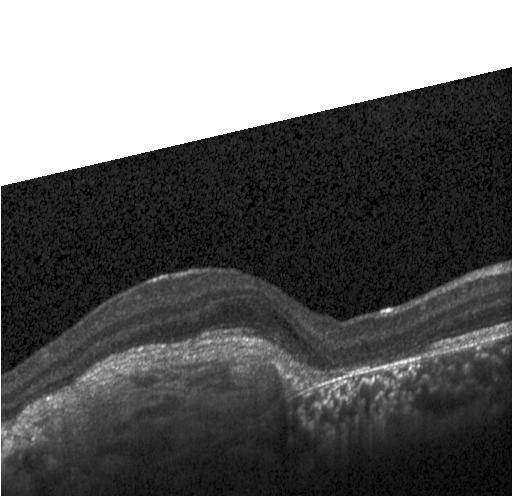
Fovea-centered; optical coherence tomography scan; spectral-domain OCT
This B-scan demonstrates choroidal neovascularization.